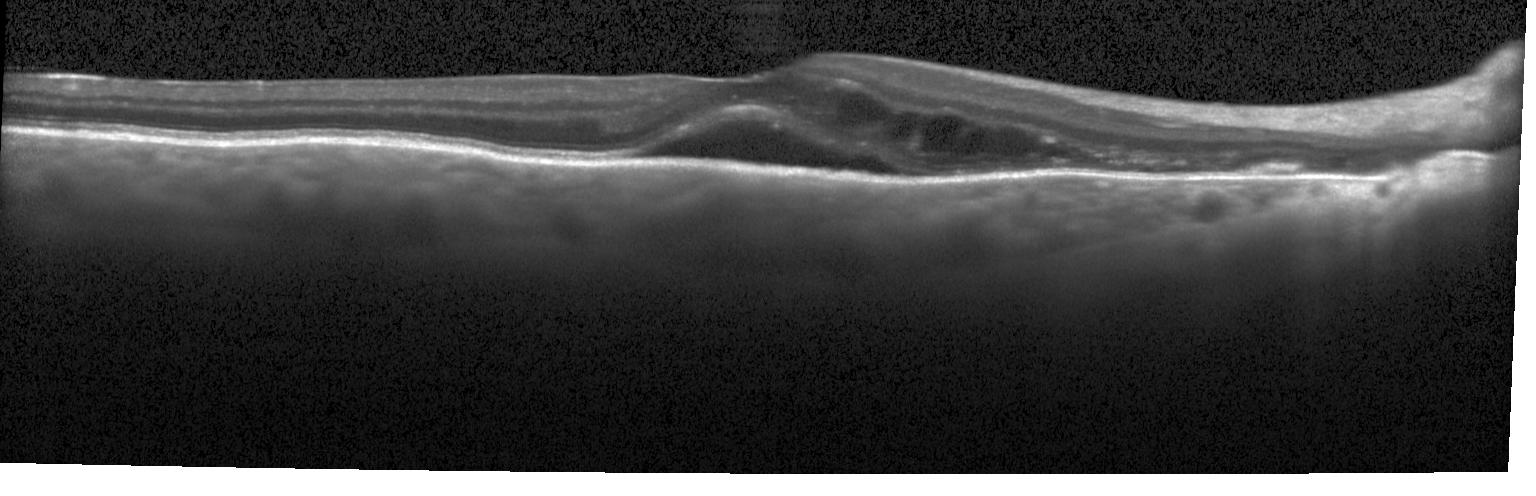

Horizontal scan through the fovea, retinal OCT cross-section, SD-OCT.
The scan shows choroidal neovascularization.